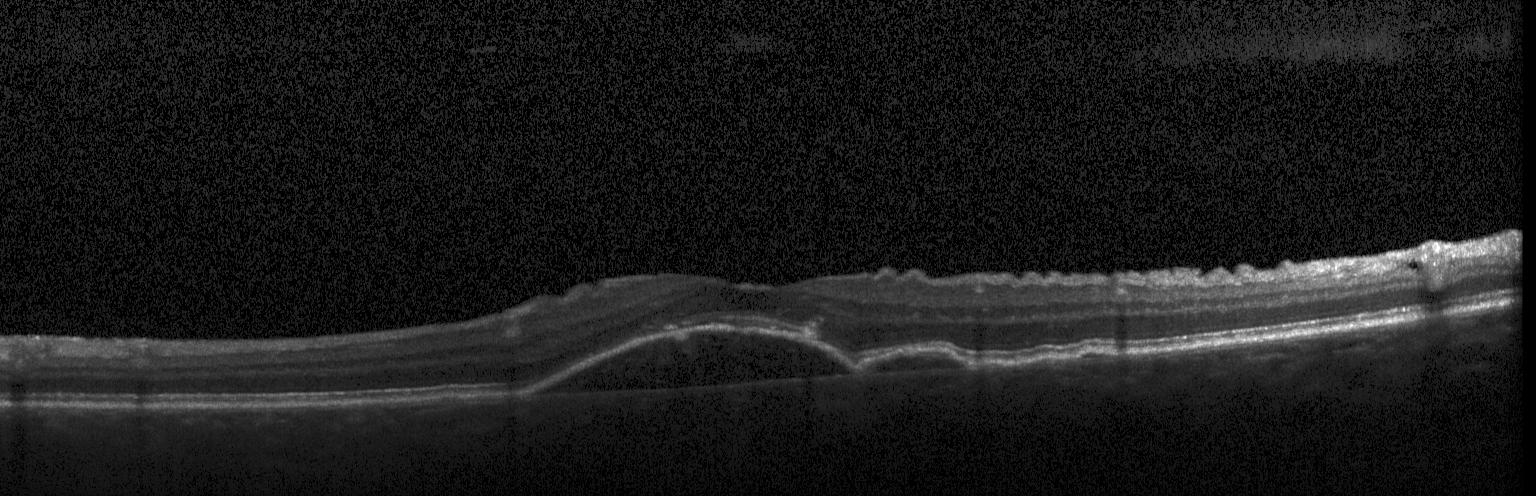

Centered on the fovea. Optical coherence tomography B-scan
Diagnosis: a choroidal neovascular membrane.